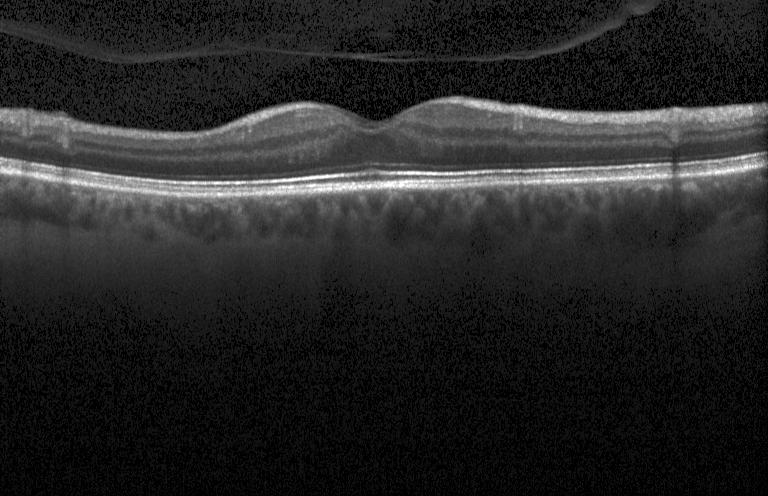

Dx: no choroidal neovascularization, no diabetic macular edema, and no drusen.